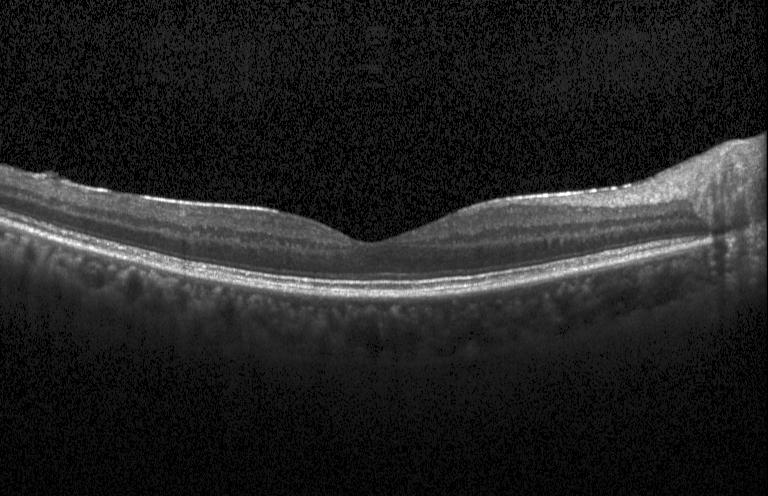
Optical coherence tomography scan.
The scan shows no evidence of choroidal neovascularization, diabetic macular edema, or drusen.